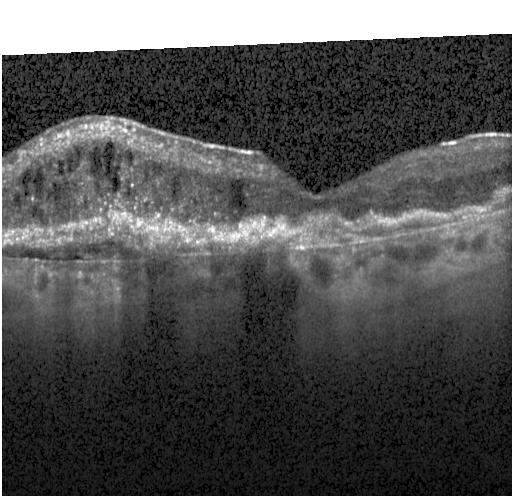
A choroidal neovascular membrane.